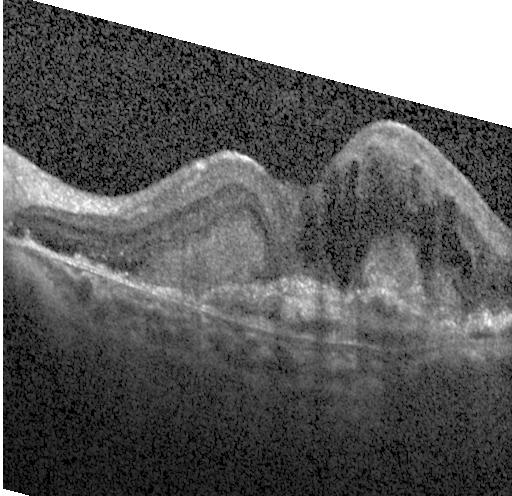

OCT finding: choroidal neovascularization (CNV).